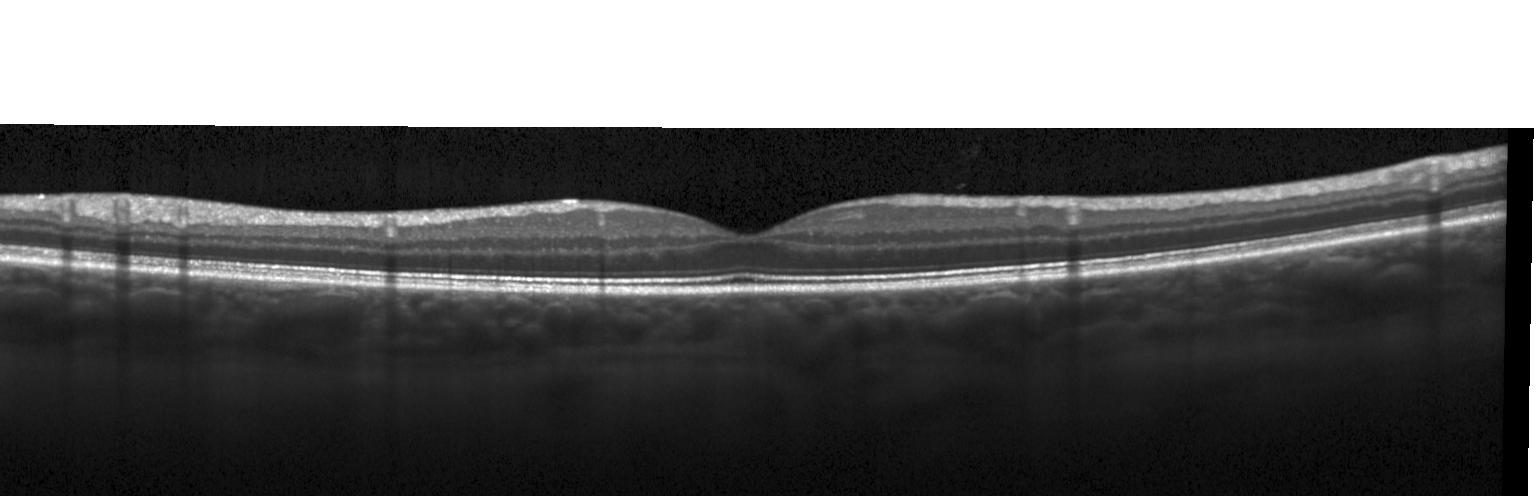

Centered on the fovea, spectral-domain OCT, optical coherence tomography B-scan
No CNV, no DME, and no drusen.